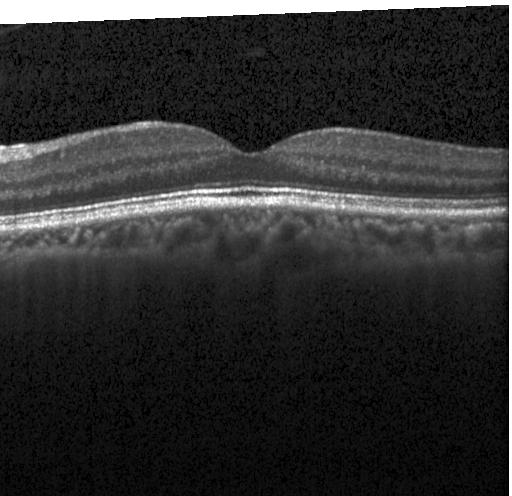

OCT B-scan — This B-scan demonstrates no evidence of choroidal neovascularization, diabetic macular edema, or drusen.